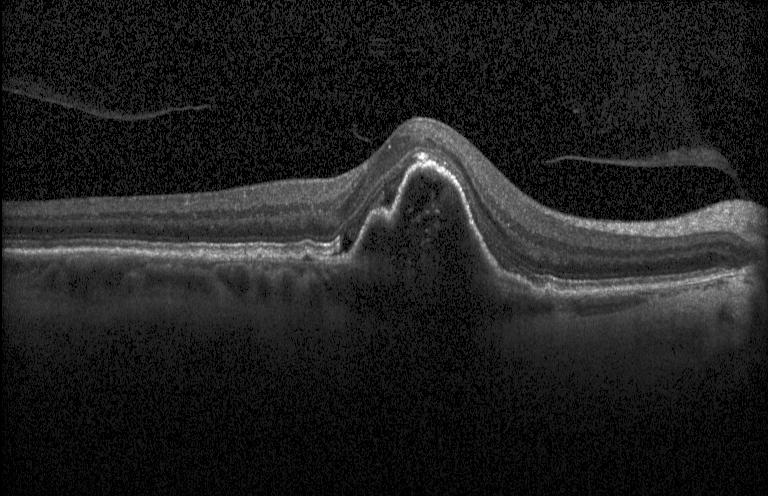

Fovea-centered · optical coherence tomography B-scan. Diagnosis: CNV.